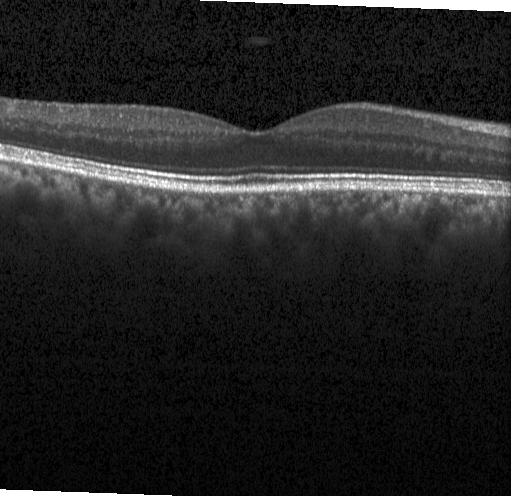

Dx: no choroidal neovascularization, no diabetic macular edema, and no drusen.